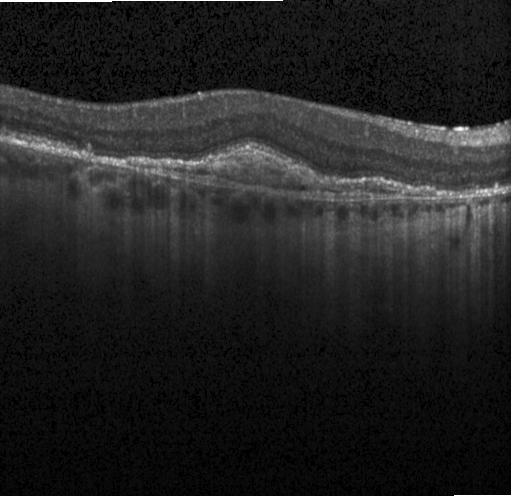 OCT line scan. Heidelberg Spectralis. The scan shows a choroidal neovascular membrane.